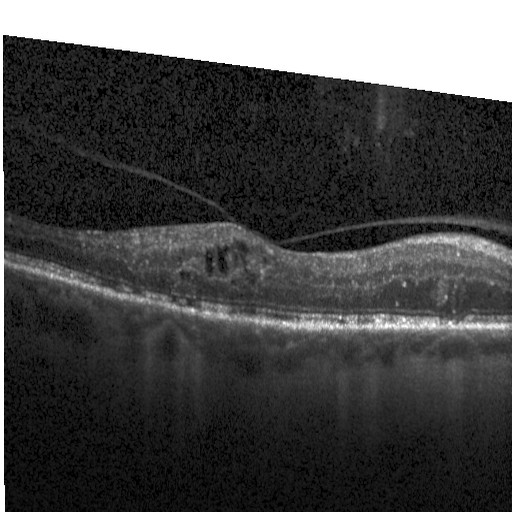 Optical coherence tomography B-scan; through the macula. Finding: diabetic macular edema.